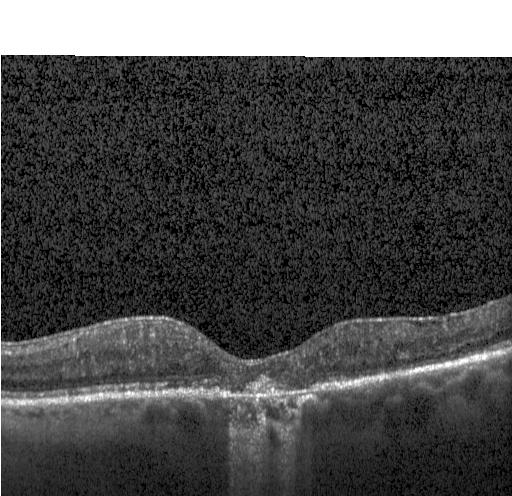
Instrument: Heidelberg Spectralis · optical coherence tomography B-scan · spectral-domain optical coherence tomography · through the macula — Choroidal neovascularization.